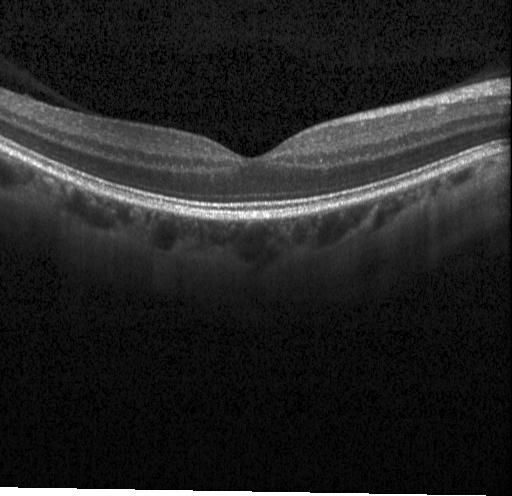

Macular scan · SD-OCT · retinal OCT cross-section · Heidelberg Spectralis.
Diagnosis: no evidence of choroidal neovascularization, diabetic macular edema, or drusen.